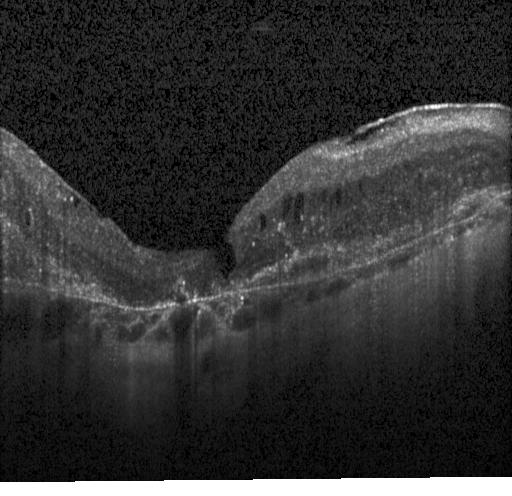 Horizontal scan through the fovea; spectral-domain optical coherence tomography; optical coherence tomography B-scan — OCT finding: a choroidal neovascular membrane.